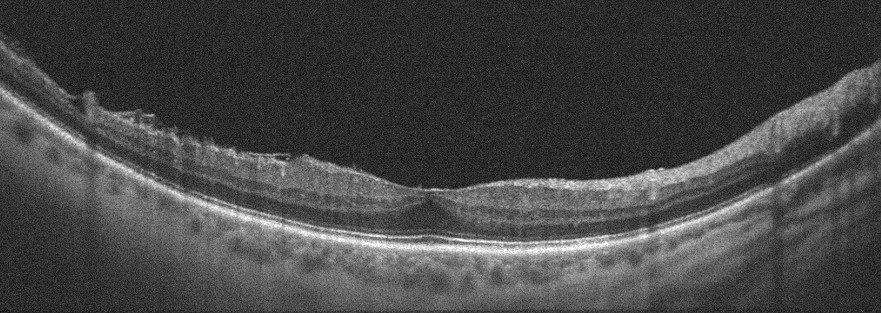 Fovea-centered; OCT line scan. Assessment: ERM.